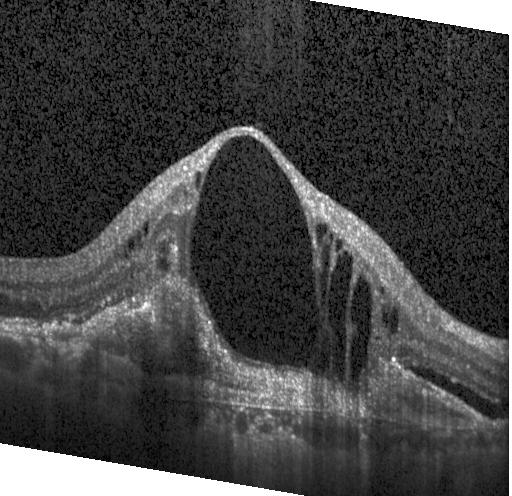
Optical coherence tomography scan, acquired on a Heidelberg Spectralis.
Assessment: a choroidal neovascular membrane.